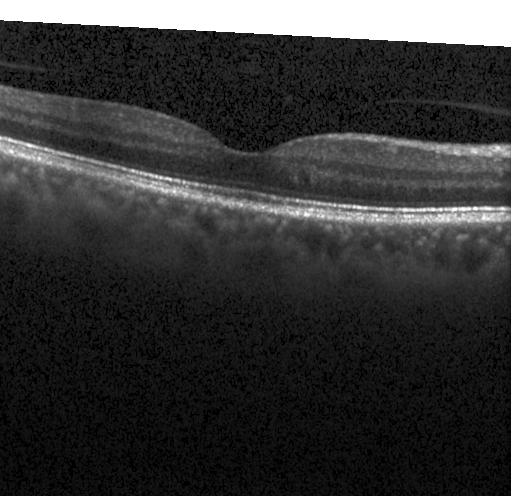

Acquired on a Heidelberg Spectralis; macular scan; SD-OCT; retinal OCT cross-section. Macular OCT: neither choroidal neovascularization, diabetic macular edema, nor drusen.